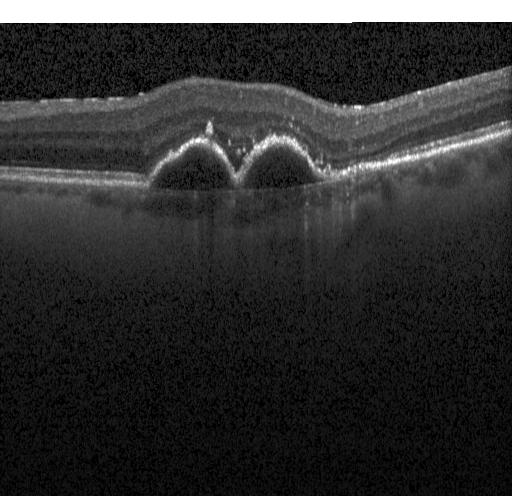

Optical coherence tomography B-scan · through the macula · Heidelberg Spectralis.
Macular OCT: CNV.